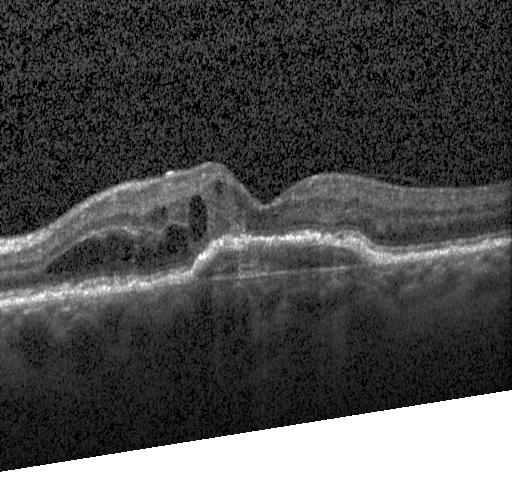

OCT B-scan · Heidelberg Spectralis. Diagnosis: a choroidal neovascular membrane.